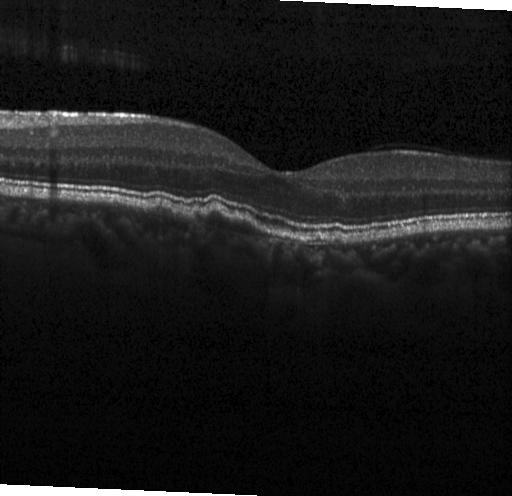 Optical coherence tomography B-scan; Heidelberg Spectralis.
Diagnosis: sub-RPE drusenoid deposits.